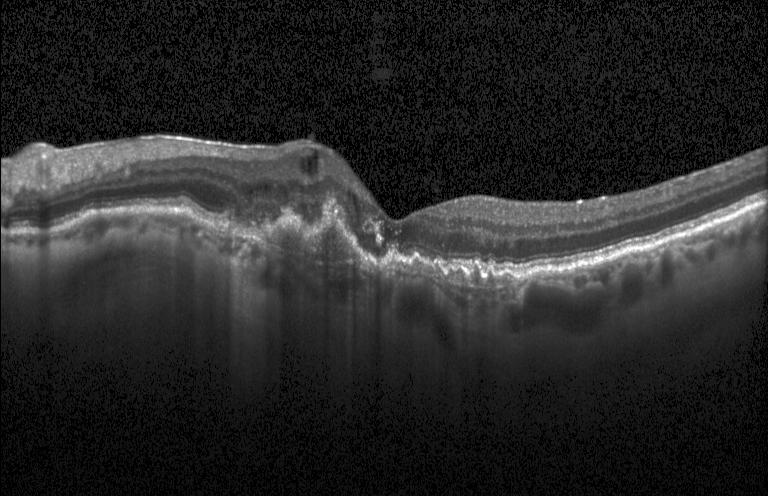
Spectral-domain OCT B-scan: choroidal neovascularization.